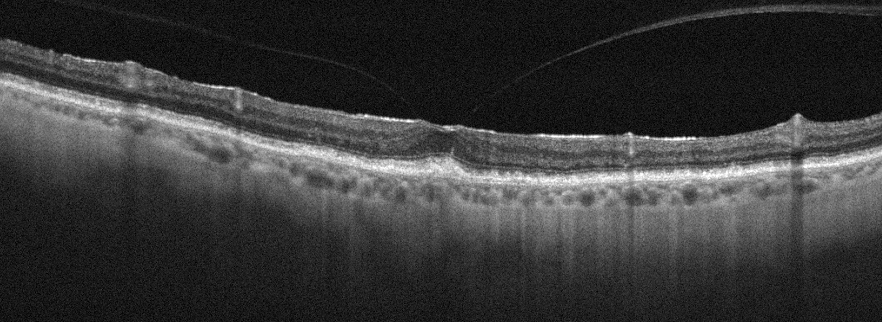

Oculus sinister, retinal OCT cross-section — Finding: VID.